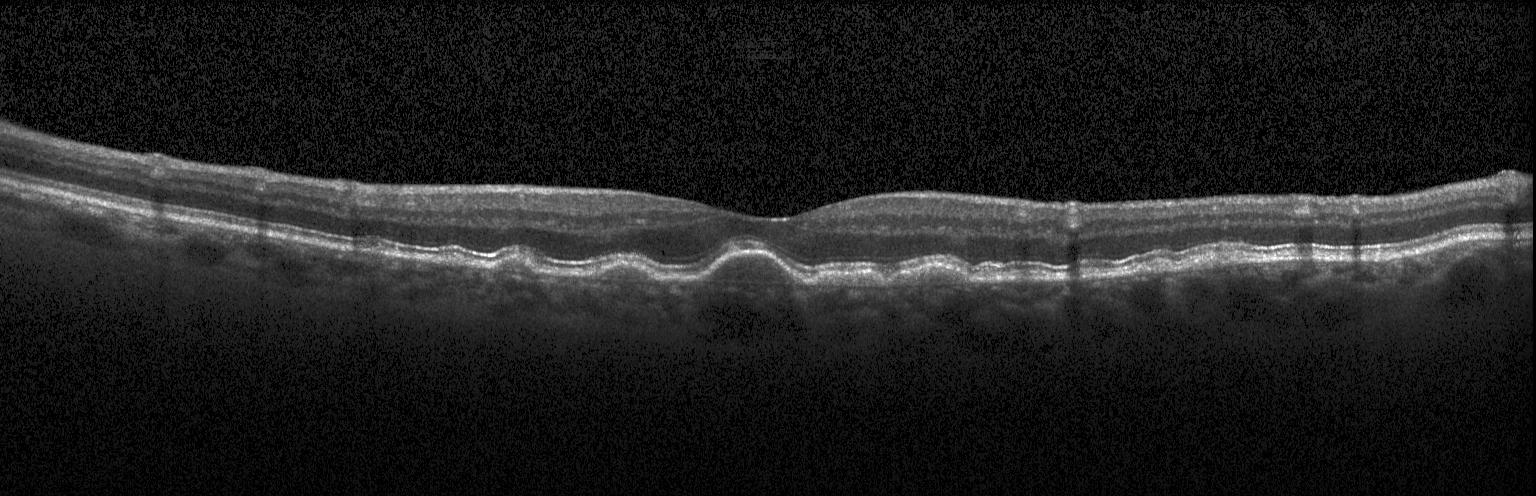
Spectral-domain optical coherence tomography; through the macula; optical coherence tomography B-scan; acquired on a Heidelberg Spectralis.
Impression: drusen.